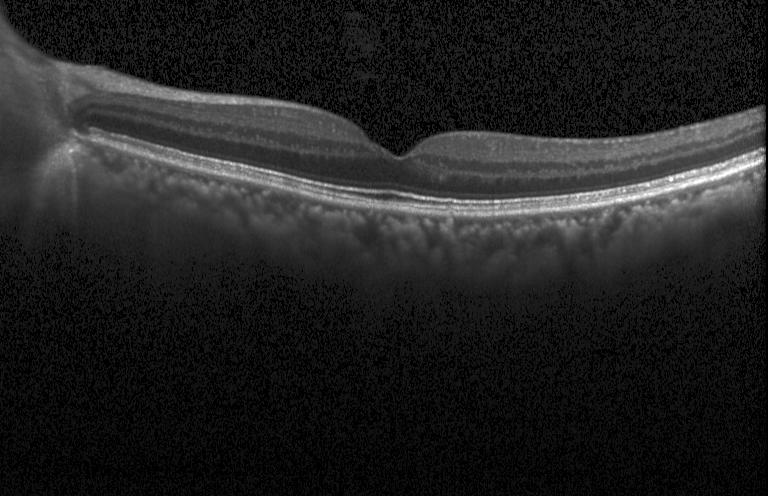

Finding: no choroidal neovascularization, diabetic macular edema, or drusen.